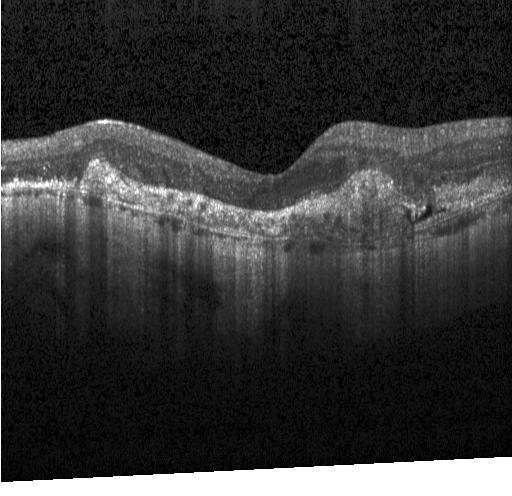 OCT scan showing choroidal neovascularization (CNV).